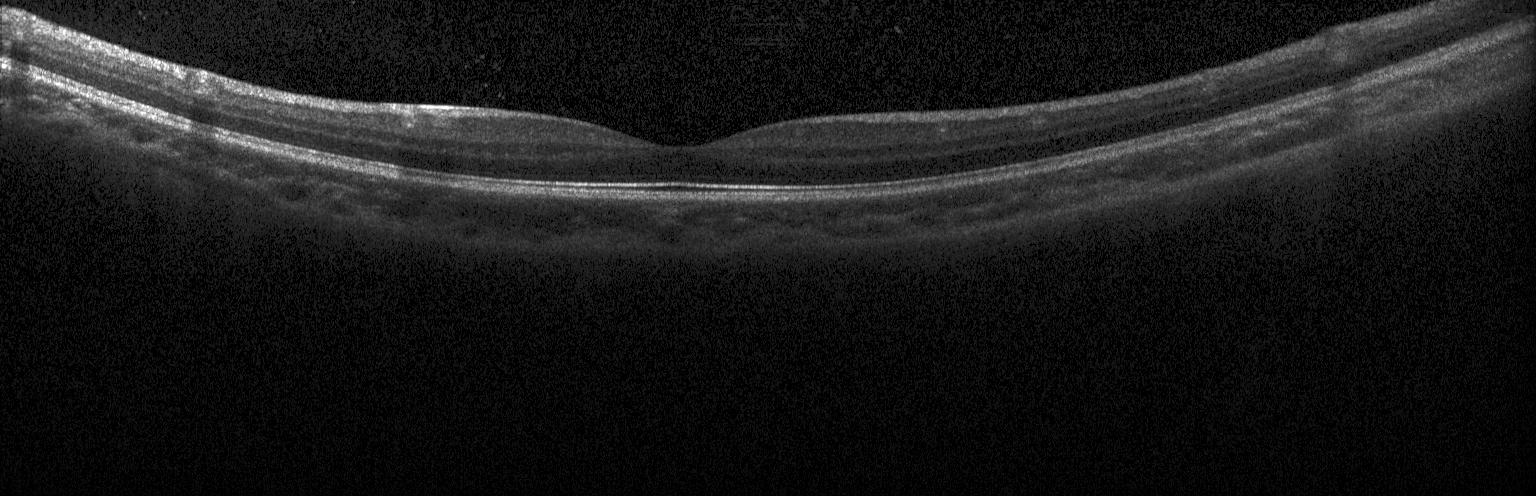

Optical coherence tomography scan
No evidence of CNV, DME, or drusen.